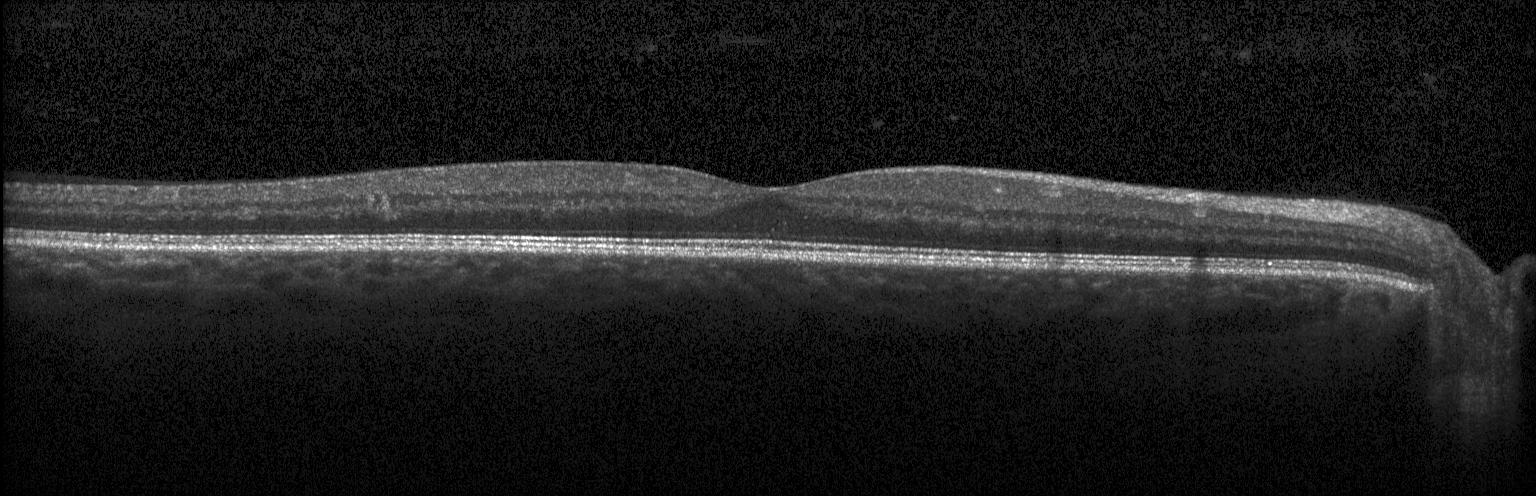 Impression: neither CNV, DME, nor drusen.